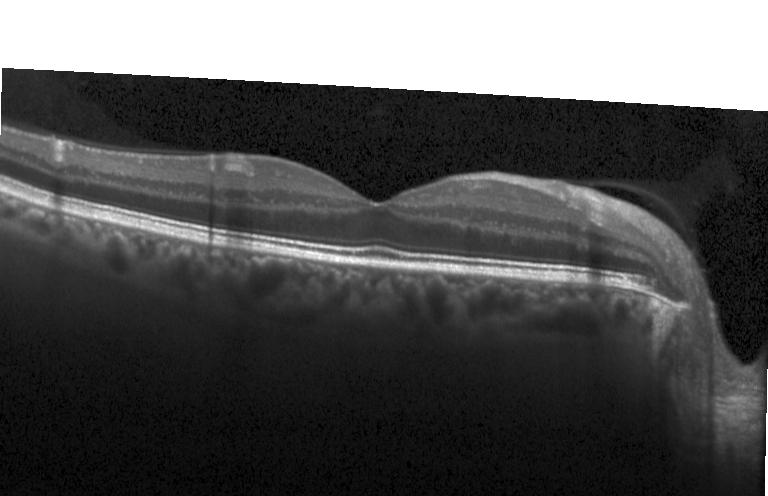
SD-OCT. Heidelberg Spectralis OCT system. Retinal OCT cross-section. No choroidal neovascularization, diabetic macular edema, or drusen.